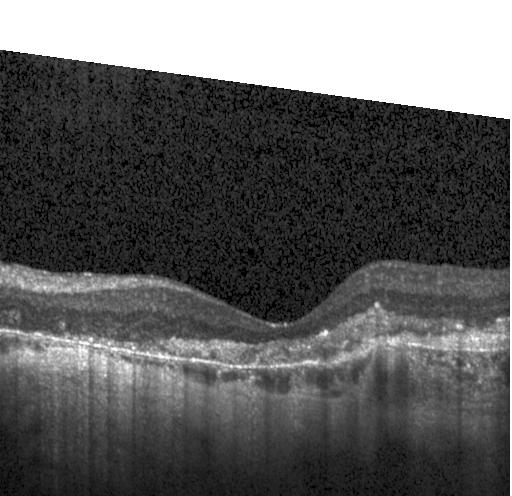

Dx: choroidal neovascularization (CNV).